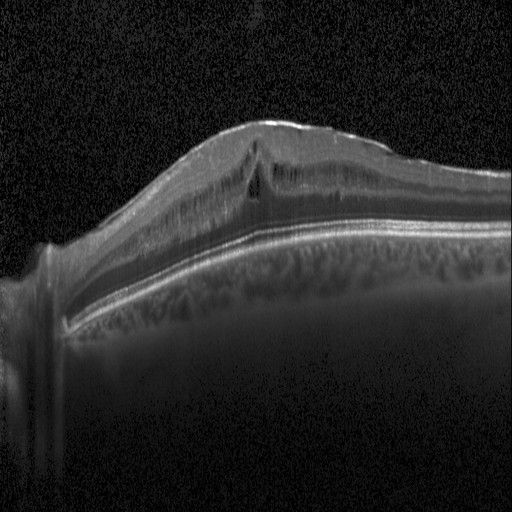

Heidelberg Spectralis, spectral-domain optical coherence tomography, optical coherence tomography scan, fovea-centered — The scan shows DME.